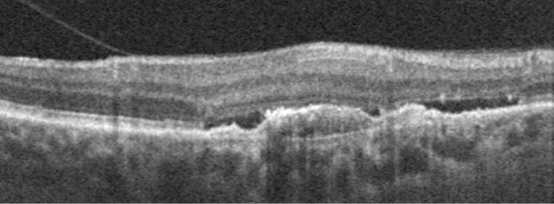

Retinal OCT cross-section, through the macula, instrument: Optovue Avanti RTVue XR.
Macular OCT: age-related macular degeneration.